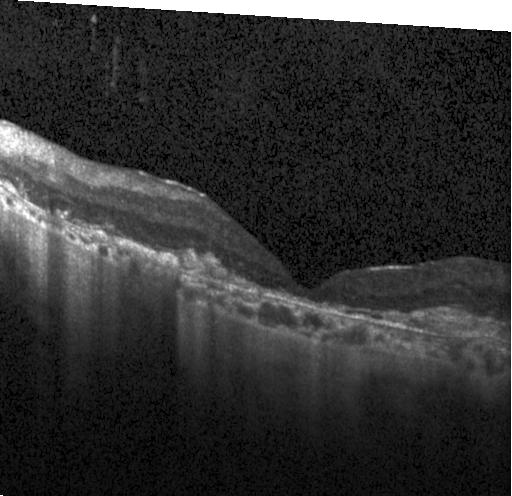 OCT finding: a choroidal neovascular membrane.